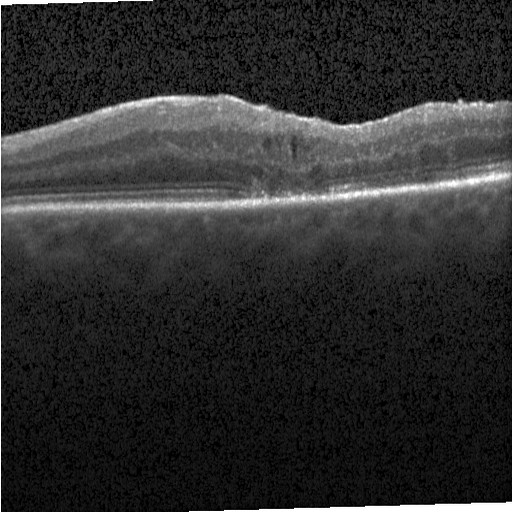
Diagnosis: DME.